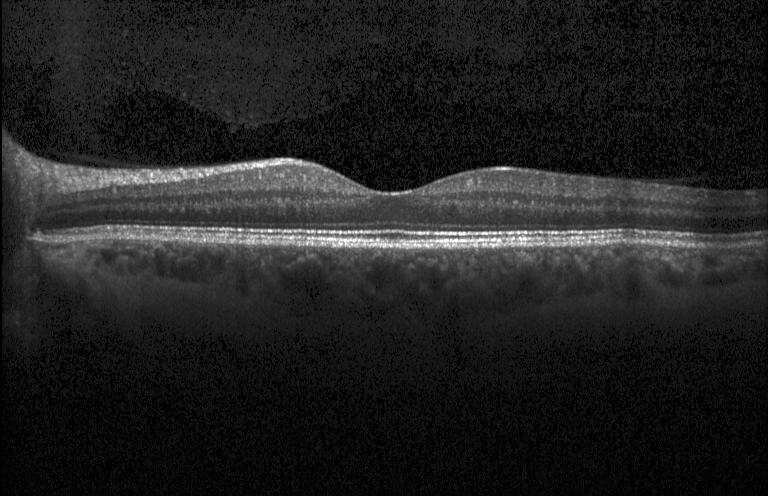

This B-scan demonstrates no CNV, DME, or drusen.